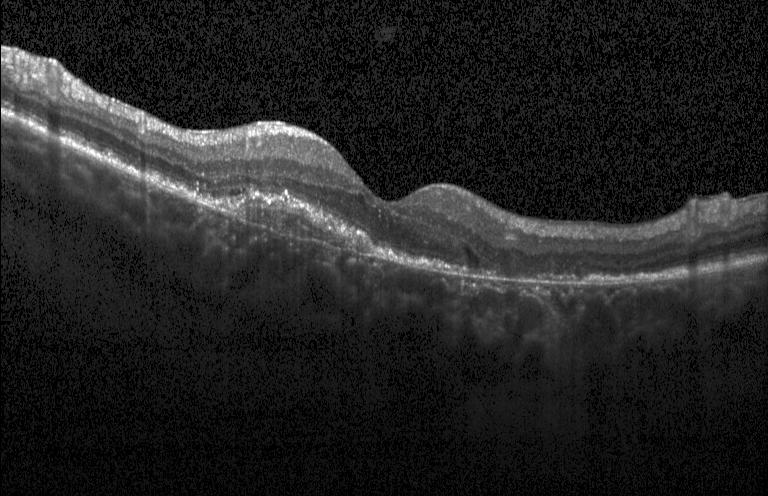
Diagnosis: a choroidal neovascular membrane.